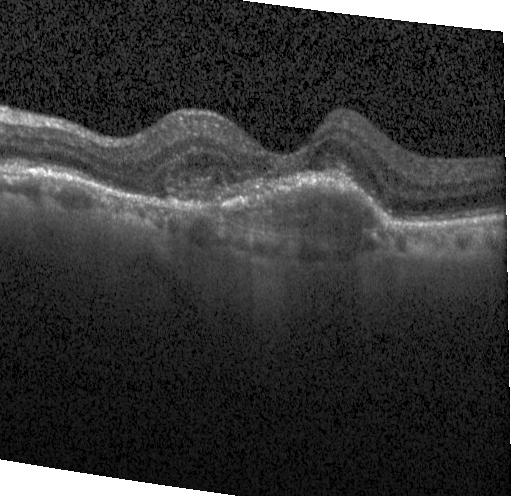 Optical coherence tomography B-scan
A choroidal neovascular membrane.